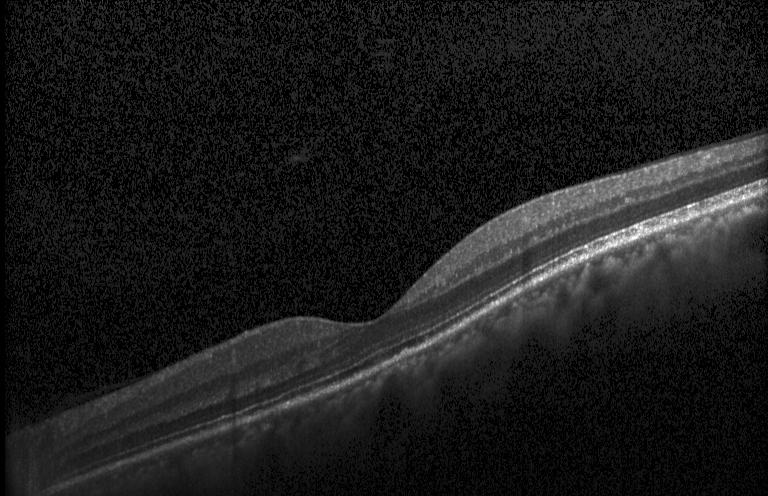

Acquired on a Heidelberg Spectralis; SD-OCT; horizontal scan through the fovea; OCT B-scan — Dx: no CNV, DME, or drusen.